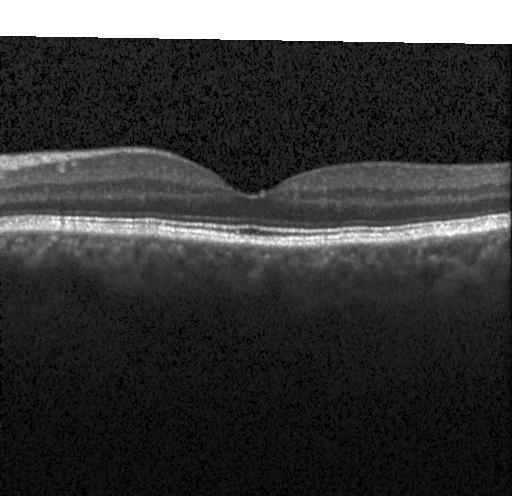 Assessment: no choroidal neovascularization, no diabetic macular edema, and no drusen.